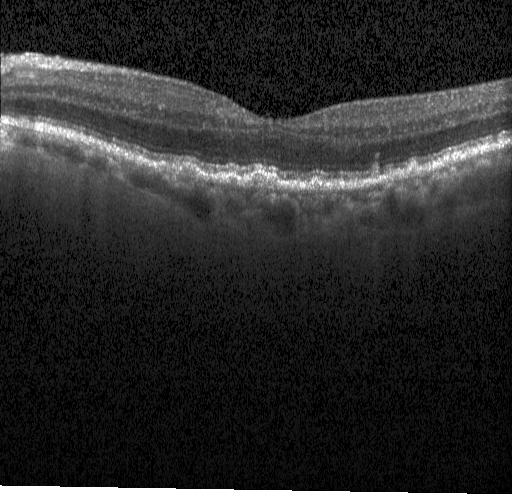

Acquired on a Heidelberg Spectralis · retinal OCT B-scan · fovea-centered · spectral-domain OCT
Diagnosis: sub-RPE drusenoid deposits.